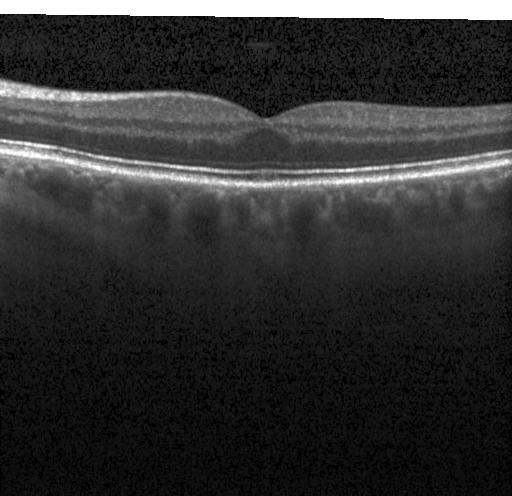

Optical coherence tomography scan. Macular scan
No choroidal neovascularization, no diabetic macular edema, and no drusen.